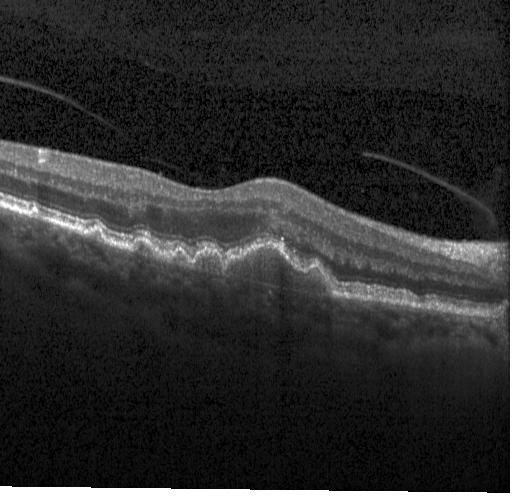

Optical coherence tomography B-scan. SD-OCT. Assessment: CNV.